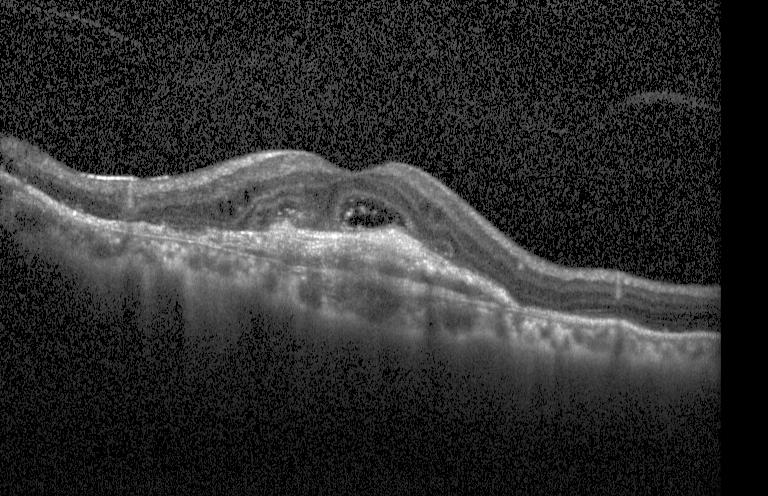
OCT B-scan.
This B-scan demonstrates choroidal neovascularization.